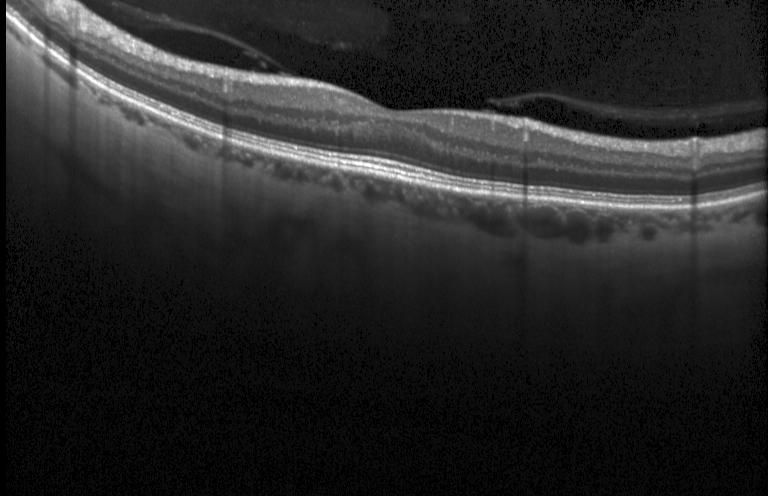

Impression: no evidence of CNV, DME, or drusen.